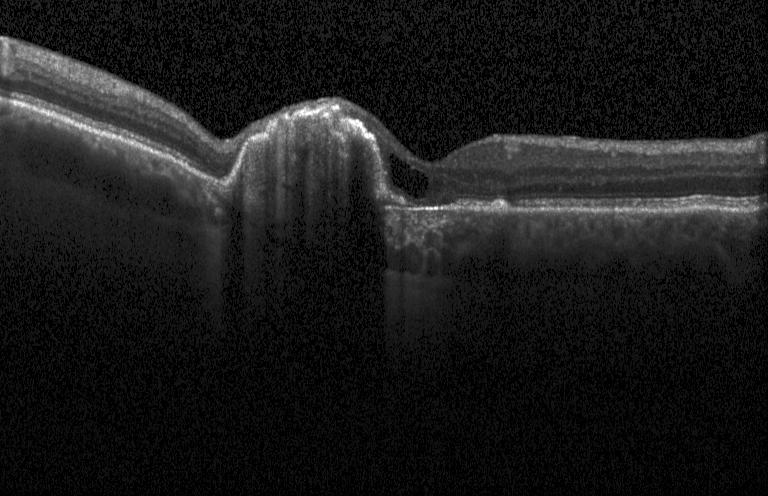 Optical coherence tomography B-scan · through the macula · spectral-domain optical coherence tomography · acquired on a Heidelberg Spectralis
Impression: choroidal neovascularization.